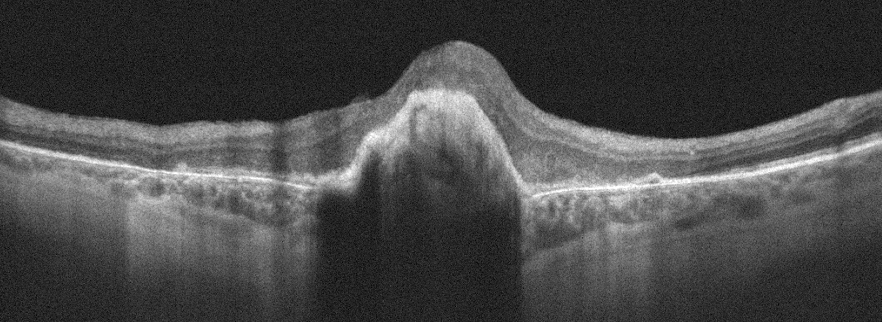

Left eye; retinal OCT cross-section. Impression: age-related macular degeneration.